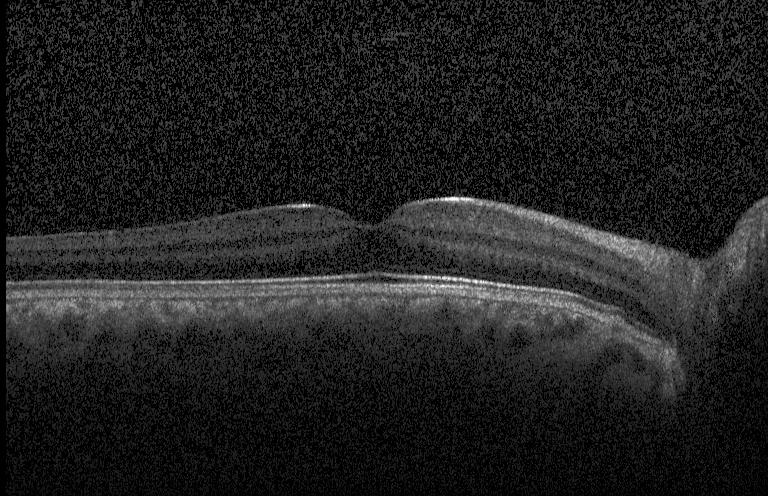
OCT finding: no CNV, no DME, and no drusen.